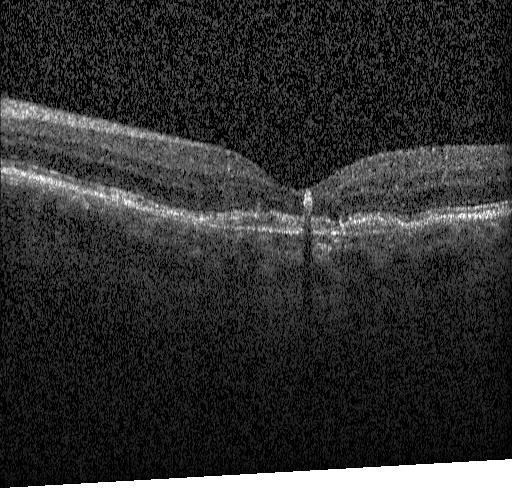 Macular OCT demonstrating a choroidal neovascular membrane.